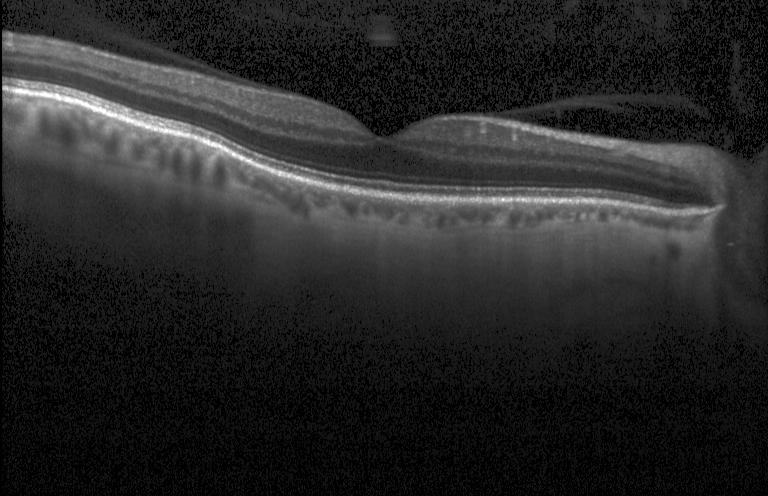
Spectral-domain OCT · acquired on a Heidelberg Spectralis · optical coherence tomography scan
Impression: no choroidal neovascularization, diabetic macular edema, or drusen.